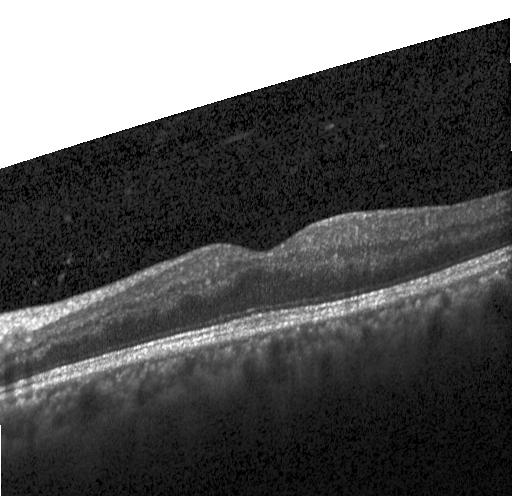

Acquired on a Heidelberg Spectralis · optical coherence tomography B-scan — Diagnosis: no evidence of choroidal neovascularization, diabetic macular edema, or drusen.